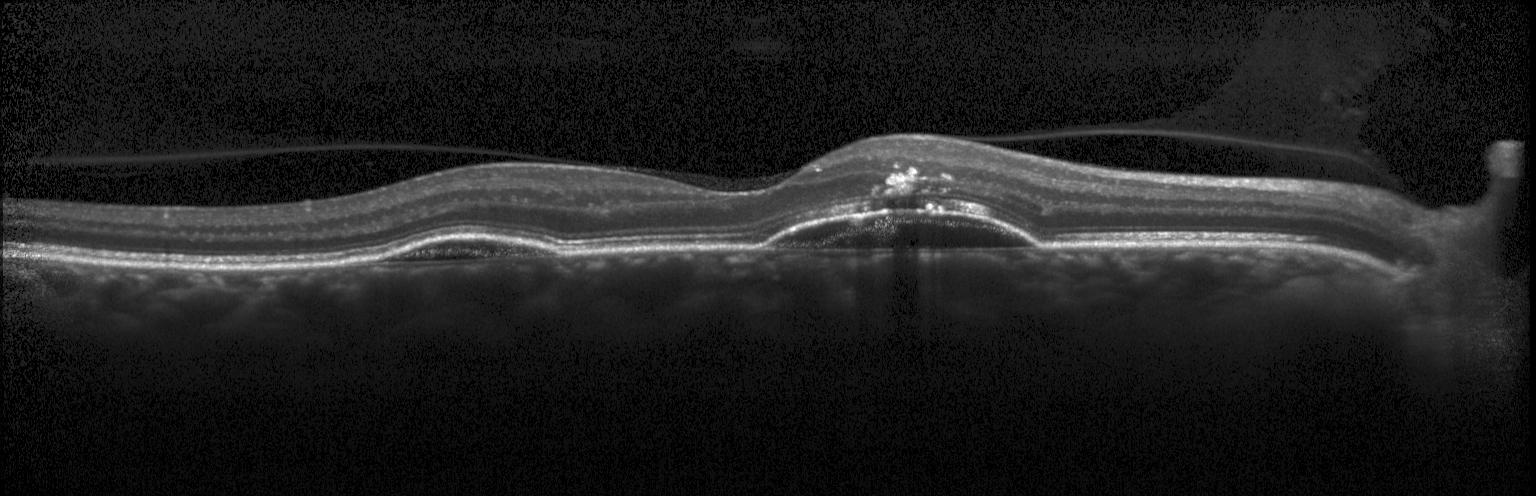 Optical coherence tomography B-scan. Spectral-domain OCT. Instrument: Heidelberg Spectralis. Through the macula. A choroidal neovascular membrane.